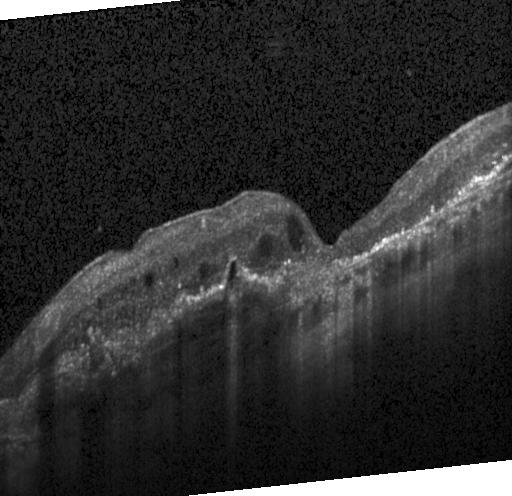

Assessment: CNV.